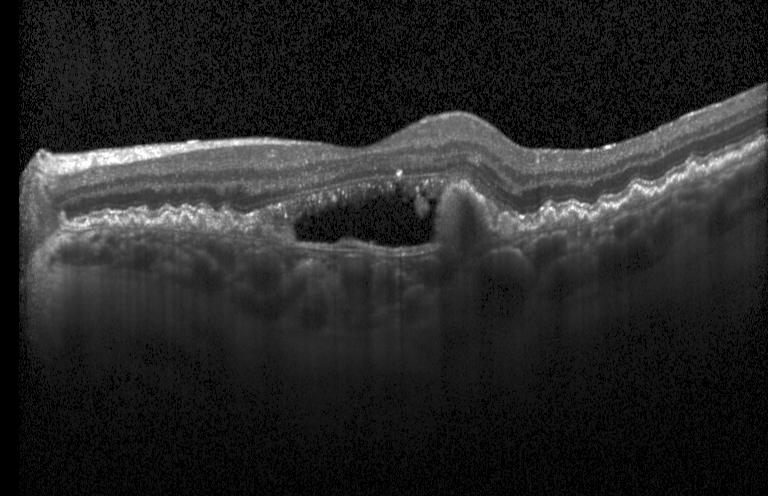

Retinal OCT B-scan · instrument: Heidelberg Spectralis.
Impression: choroidal neovascularization.